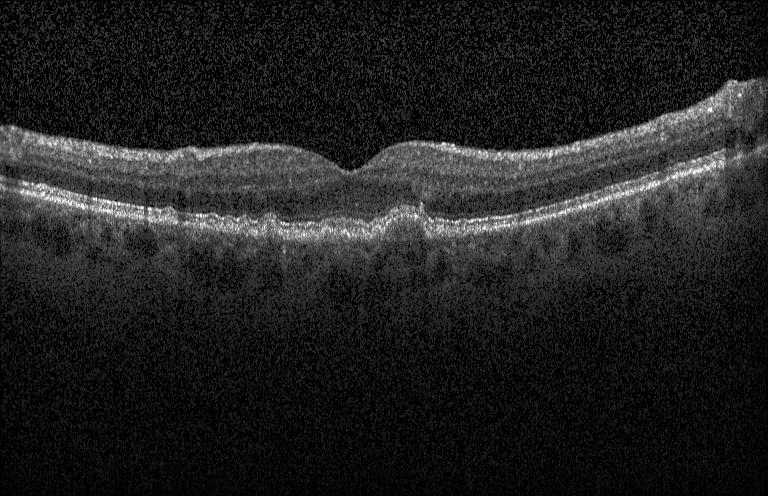
Impression: multiple drusen.